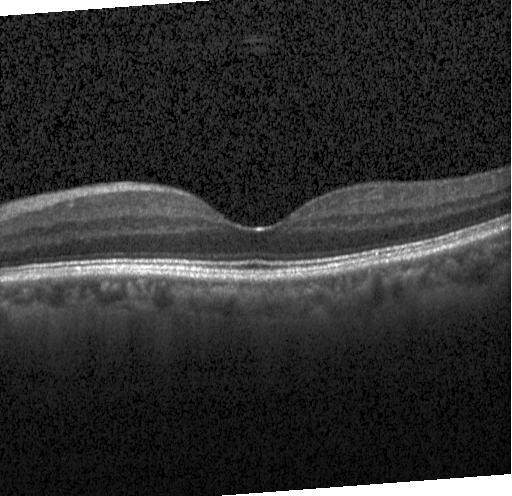

Dx: neither choroidal neovascularization, diabetic macular edema, nor drusen.